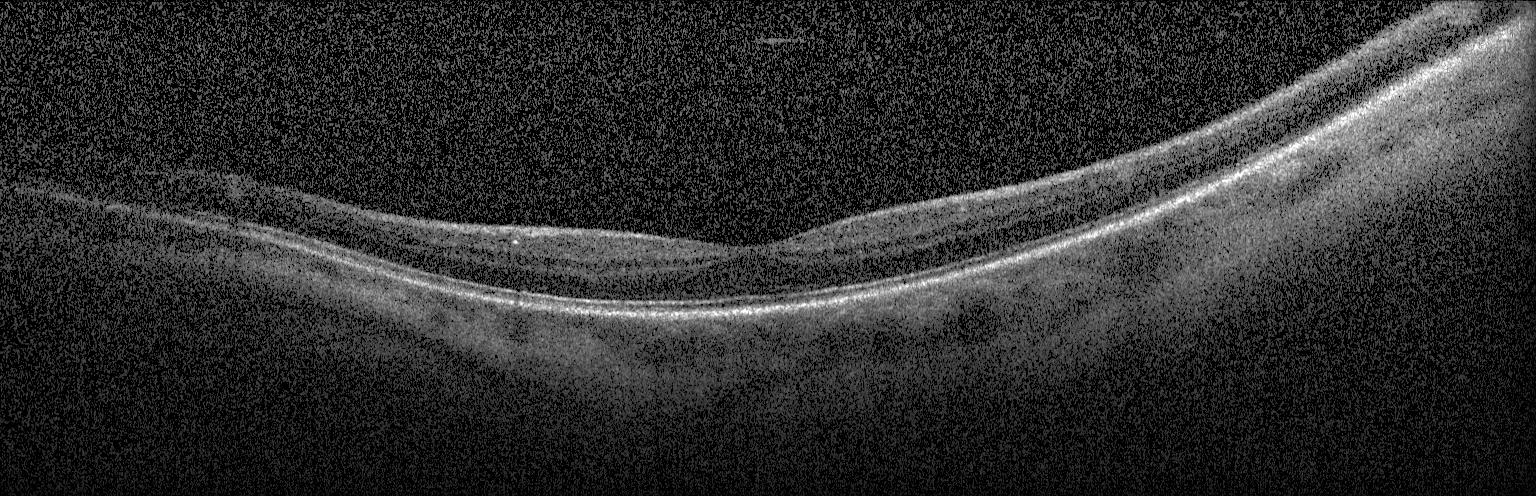 Finding: no evidence of CNV, DME, or drusen.